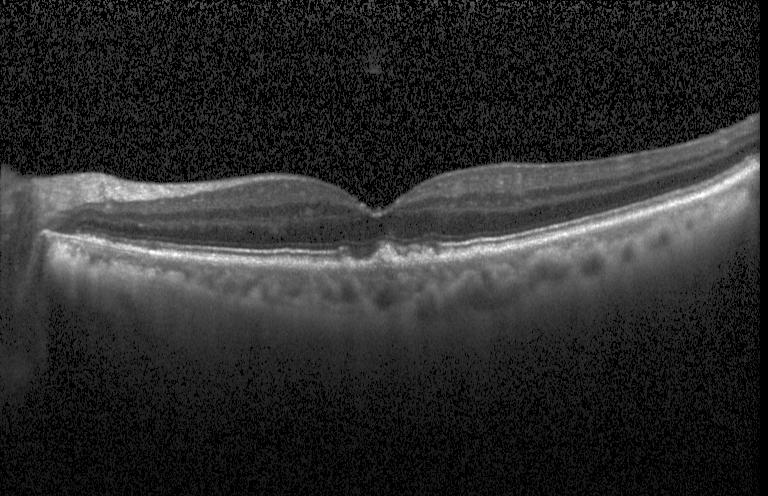 Acquired on a Heidelberg Spectralis, retinal OCT cross-section. Diagnosis: sub-RPE drusenoid deposits.